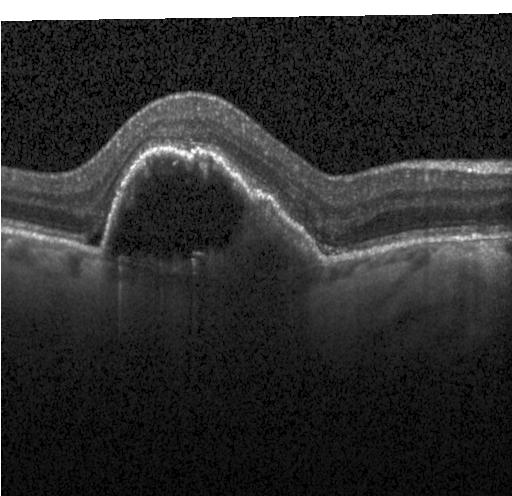
Optical coherence tomography scan — Finding: choroidal neovascularization (CNV).